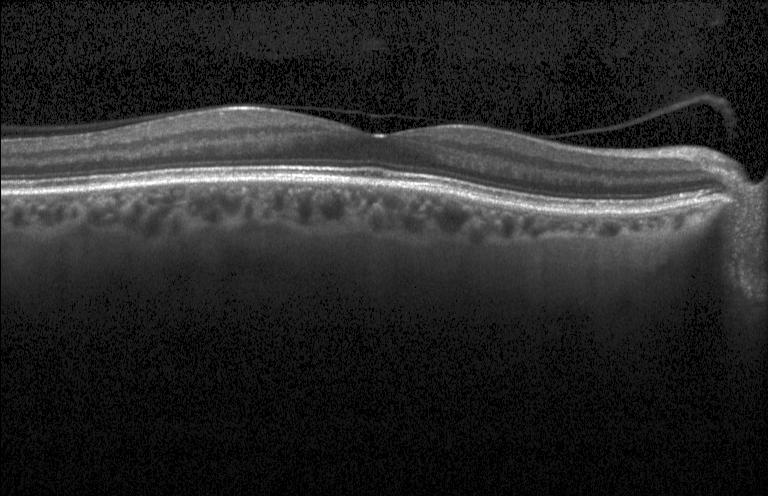

Centered on the fovea, SD-OCT, retinal OCT cross-section, instrument: Heidelberg Spectralis.
Finding: no choroidal neovascularization, no diabetic macular edema, and no drusen.